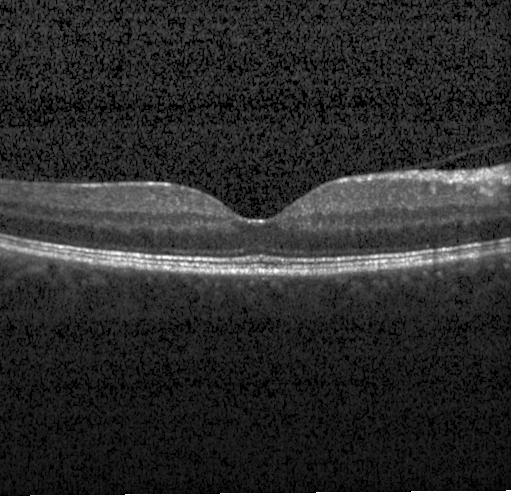 The scan shows no choroidal neovascularization, diabetic macular edema, or drusen.